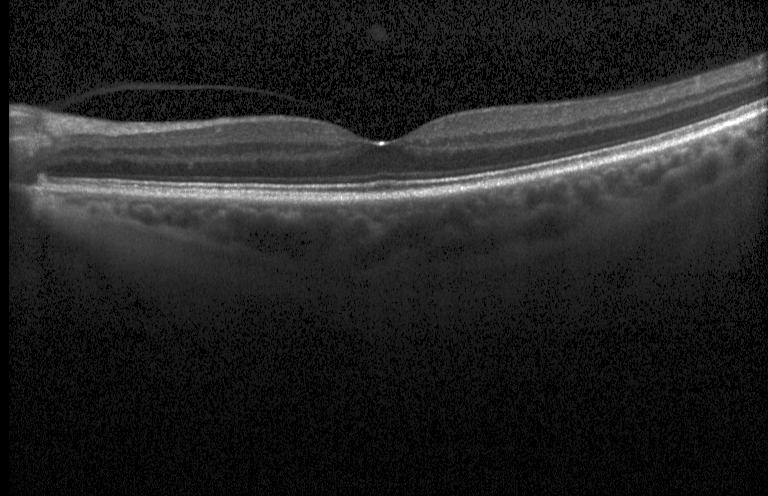 Horizontal scan through the fovea. Instrument: Heidelberg Spectralis. Optical coherence tomography scan. OCT finding: neither choroidal neovascularization, diabetic macular edema, nor drusen.